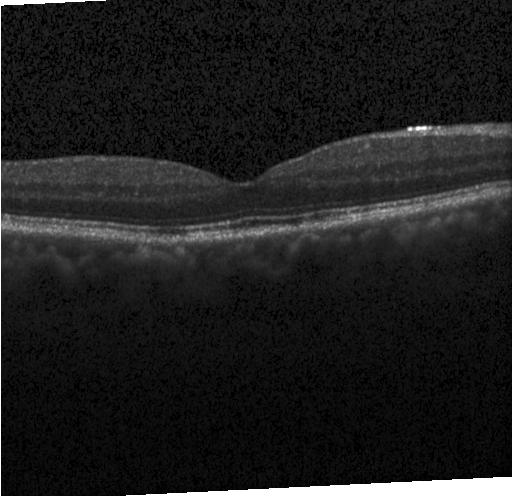 Diagnosis: no CNV, DME, or drusen.